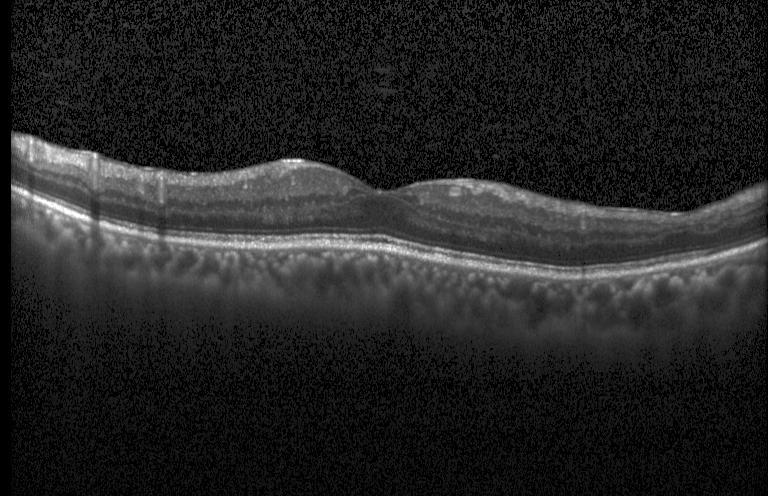
Macular scan, retinal OCT B-scan. Finding: no evidence of CNV, DME, or drusen.